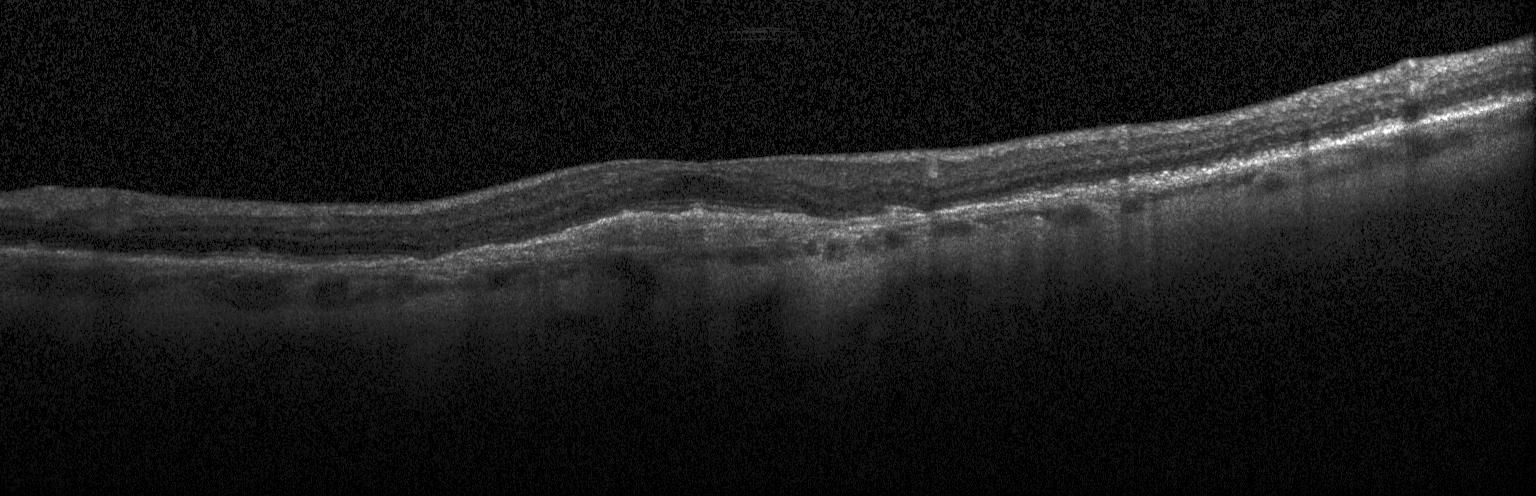

Retinal OCT cross-section showing a choroidal neovascular membrane.